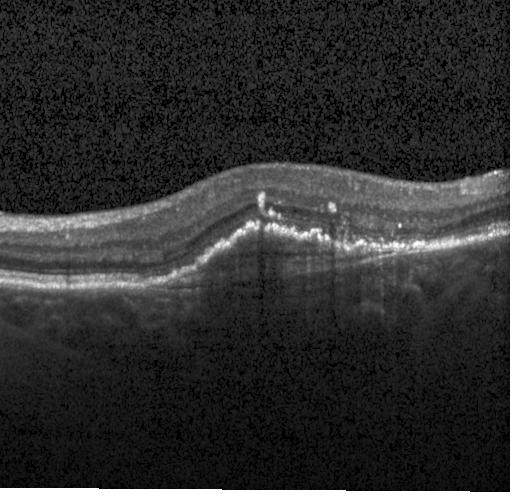

The scan shows a choroidal neovascular membrane.